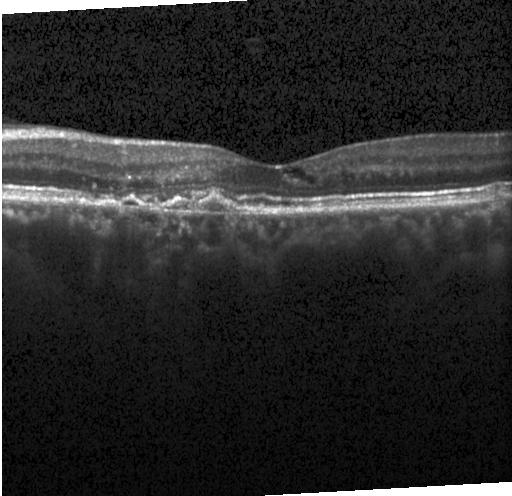
Acquired on a Heidelberg Spectralis; retinal OCT B-scan. Macular OCT: choroidal neovascularization (CNV).